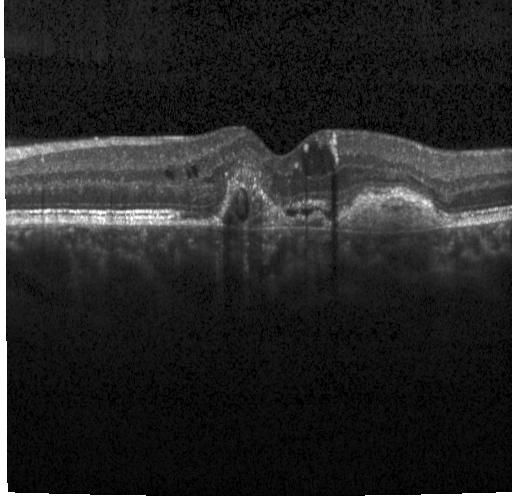
OCT B-scan showing choroidal neovascularization.